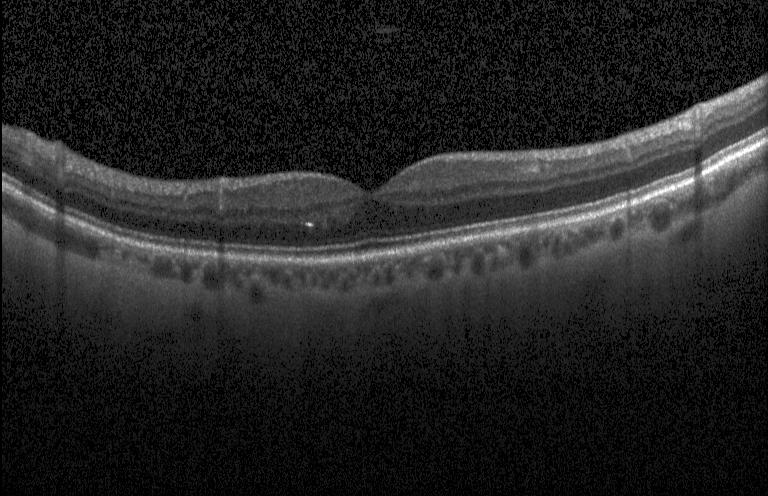
Optical coherence tomography scan. Dx: no choroidal neovascularization, no diabetic macular edema, and no drusen.